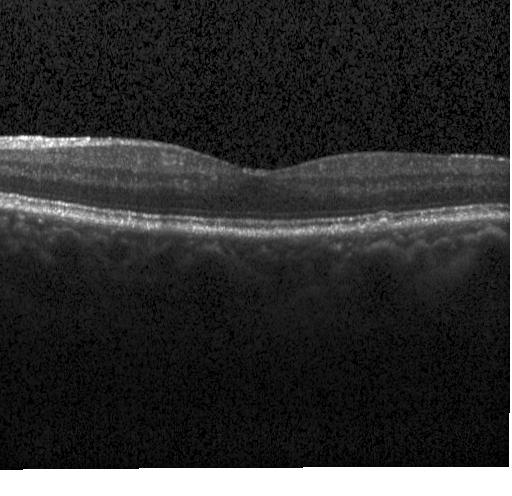

Diagnosis: drusen.